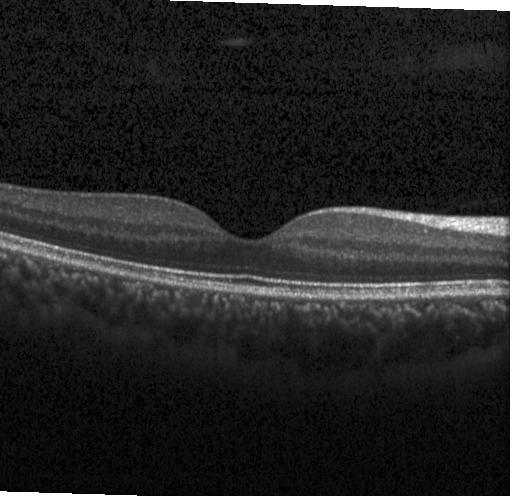 Finding: no choroidal neovascularization, diabetic macular edema, or drusen.